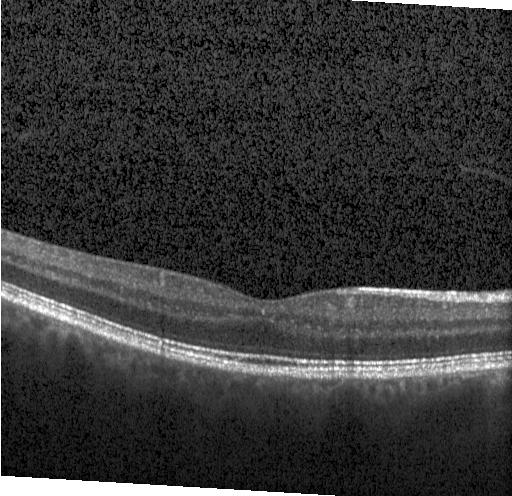 Impression: no choroidal neovascularization, diabetic macular edema, or drusen.